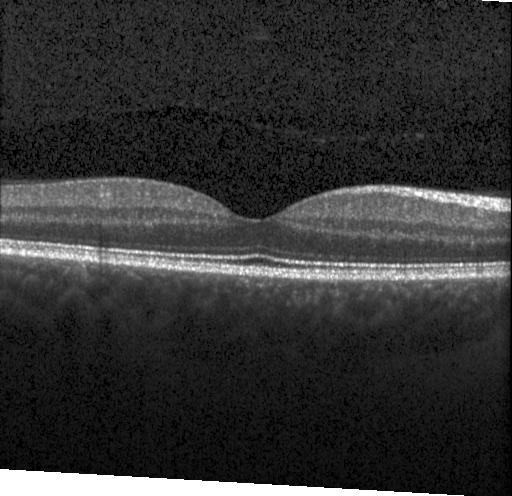
Finding: no CNV, DME, or drusen.